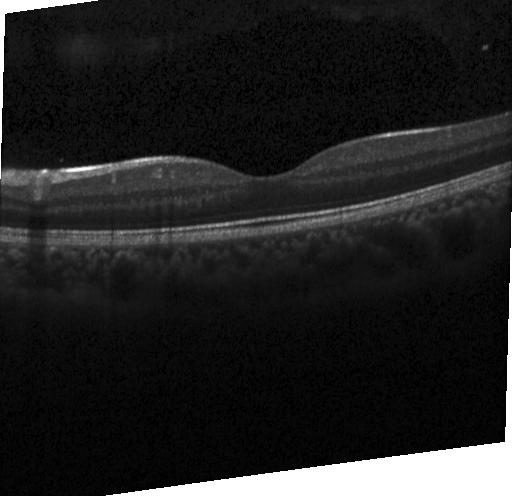
OCT finding: no choroidal neovascularization, no diabetic macular edema, and no drusen.